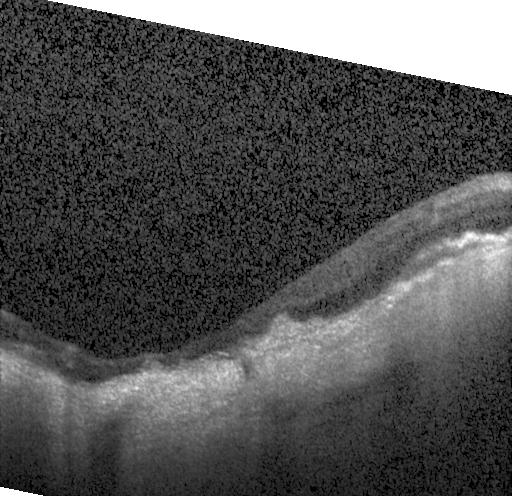

Macular scan; spectral-domain OCT; optical coherence tomography B-scan; Heidelberg Spectralis OCT system — Assessment: a choroidal neovascular membrane.